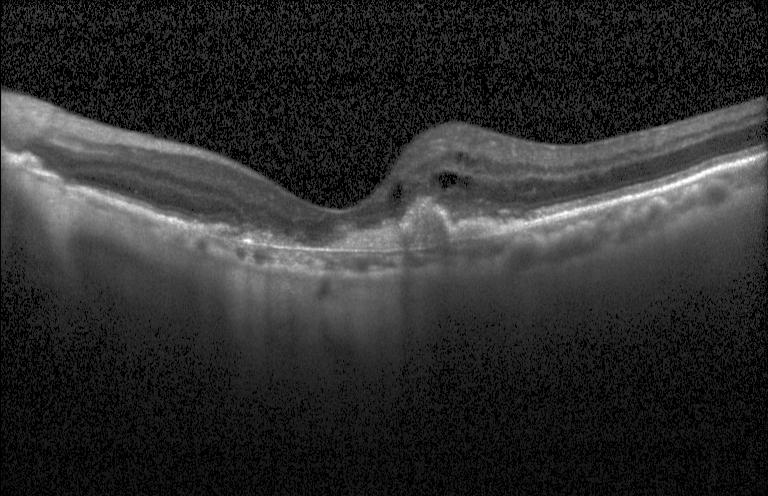 Through the macula · OCT B-scan — This B-scan demonstrates a choroidal neovascular membrane.